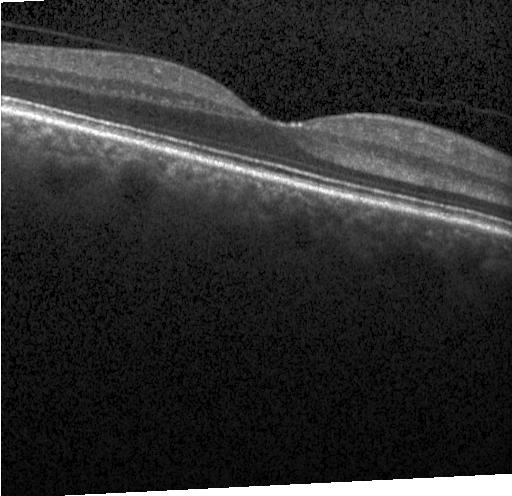 Optical coherence tomography scan; spectral-domain OCT. Impression: no choroidal neovascularization, diabetic macular edema, or drusen.